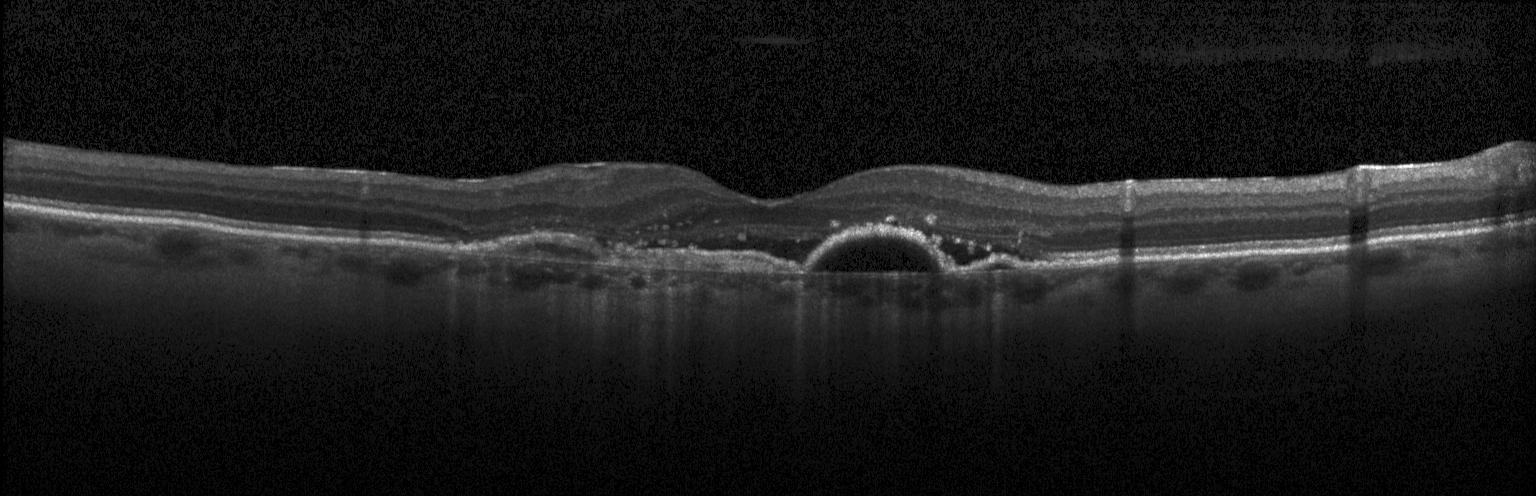
Diagnosis: choroidal neovascularization.